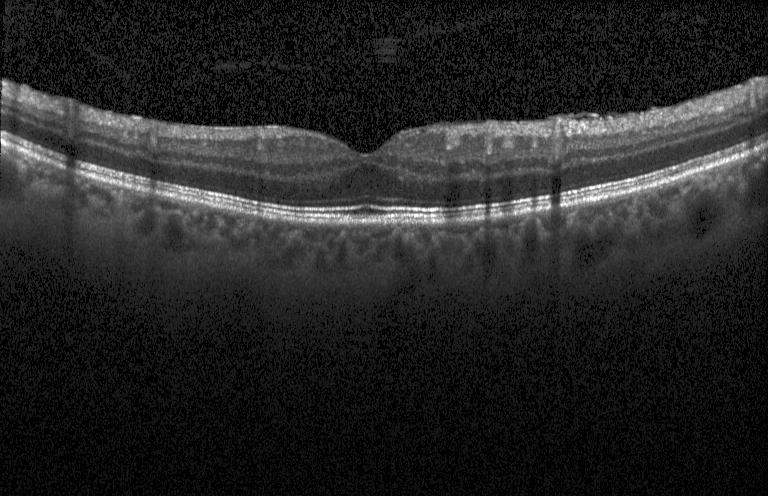
Macular OCT: no choroidal neovascularization, diabetic macular edema, or drusen.